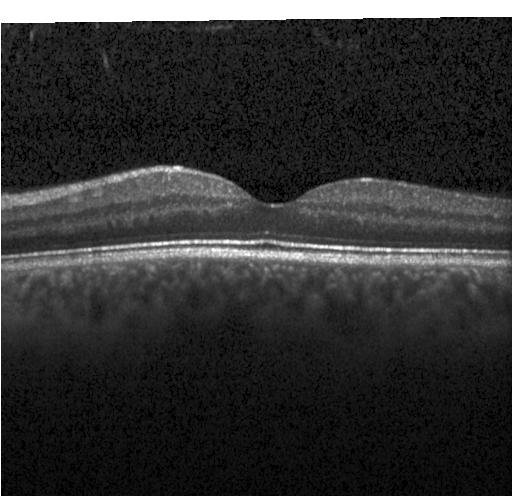

Spectral-domain optical coherence tomography · Heidelberg Spectralis · fovea-centered · optical coherence tomography B-scan
Diagnosis: no evidence of choroidal neovascularization, diabetic macular edema, or drusen.